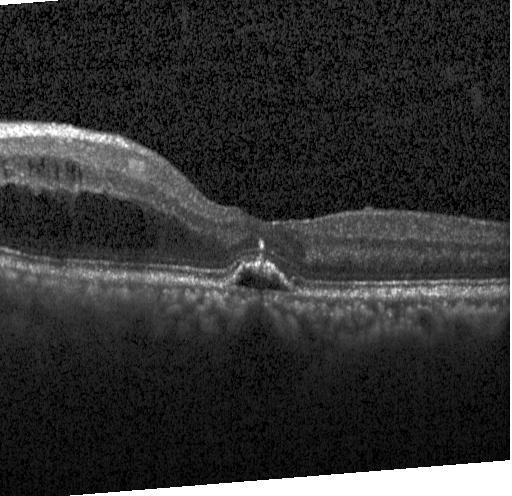

OCT B-scan.
Finding: CNV.